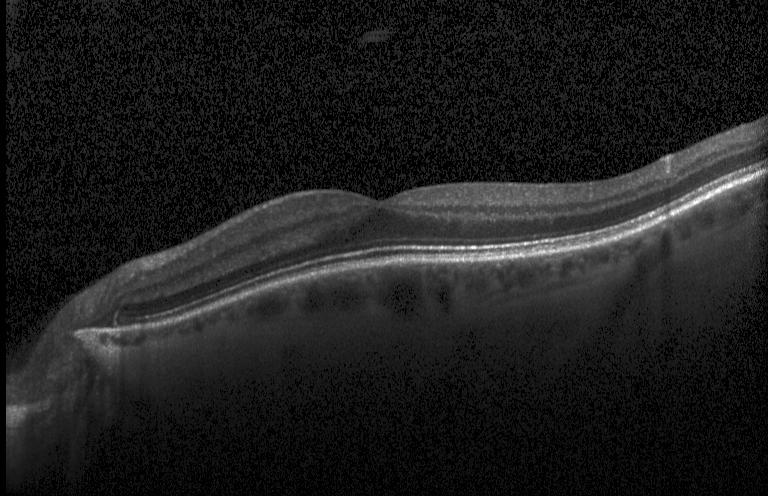 Instrument: Heidelberg Spectralis; retinal OCT B-scan — Finding: no choroidal neovascularization, diabetic macular edema, or drusen.